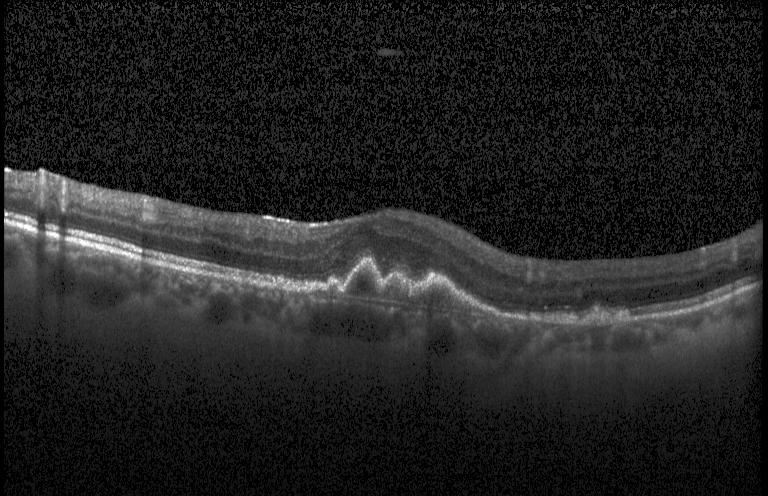 SD-OCT · Heidelberg Spectralis OCT system · optical coherence tomography scan — The scan shows a choroidal neovascular membrane.